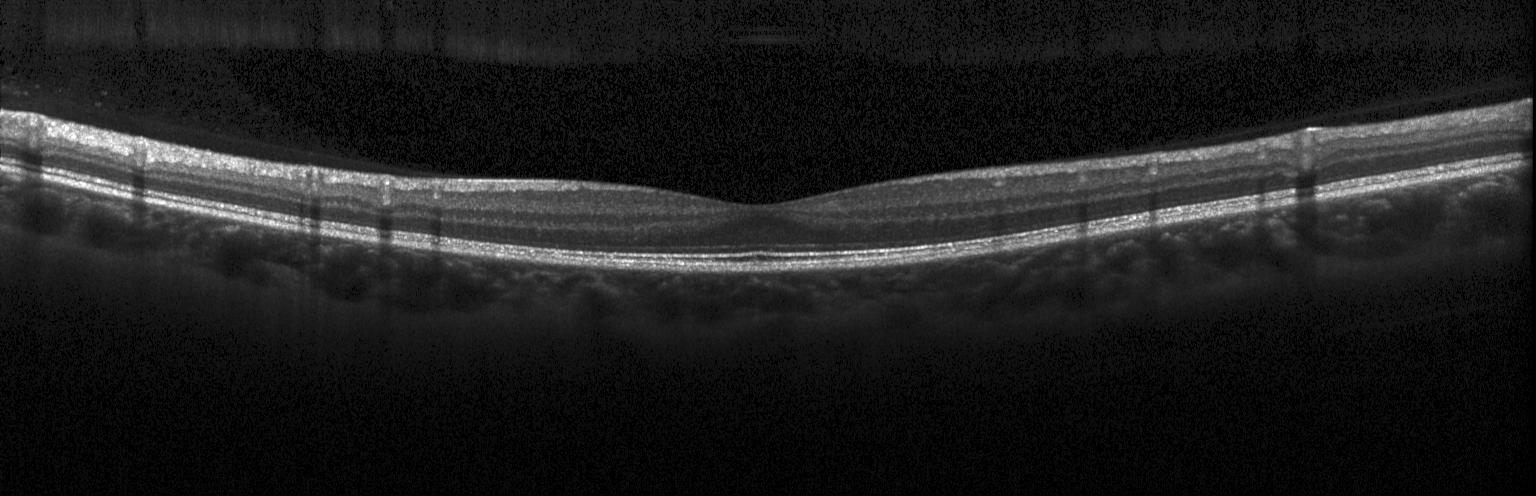
Diagnosis: no evidence of choroidal neovascularization, diabetic macular edema, or drusen.